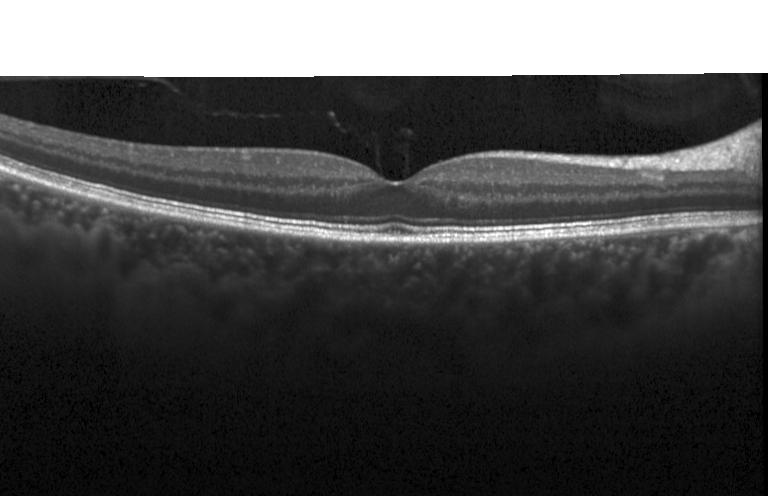
OCT B-scan
This B-scan demonstrates neither choroidal neovascularization, diabetic macular edema, nor drusen.